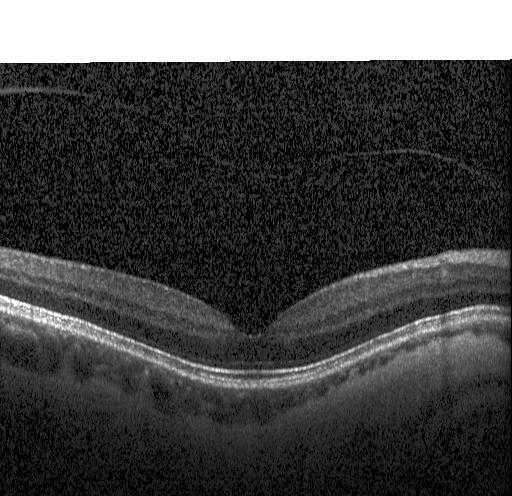 Impression: no choroidal neovascularization, diabetic macular edema, or drusen.